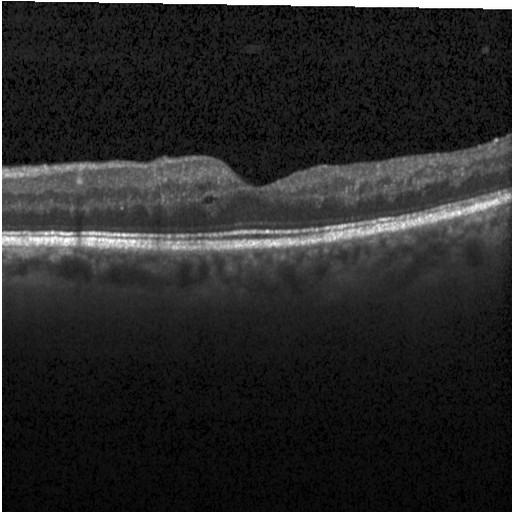

Spectral-domain OCT, optical coherence tomography B-scan, instrument: Heidelberg Spectralis
Dx: diabetic macular edema (DME).